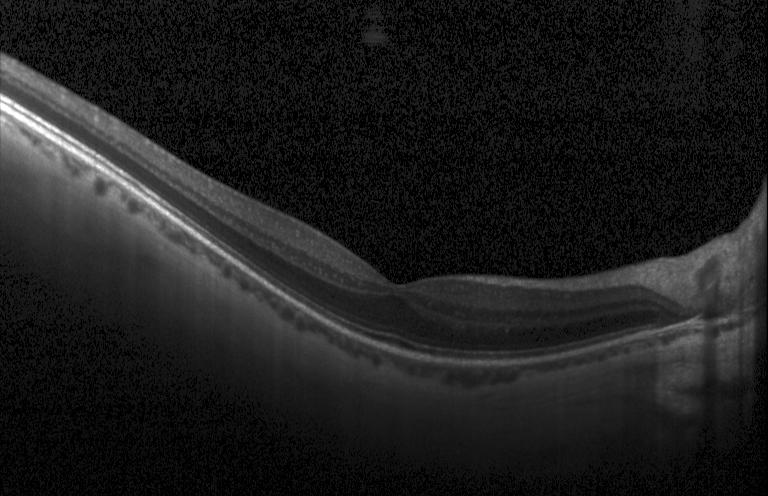 Retinal OCT cross-section showing neither choroidal neovascularization, diabetic macular edema, nor drusen.